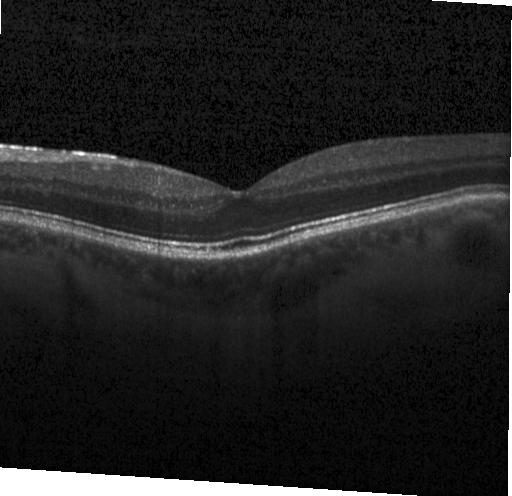 Macular OCT: no evidence of choroidal neovascularization, diabetic macular edema, or drusen.